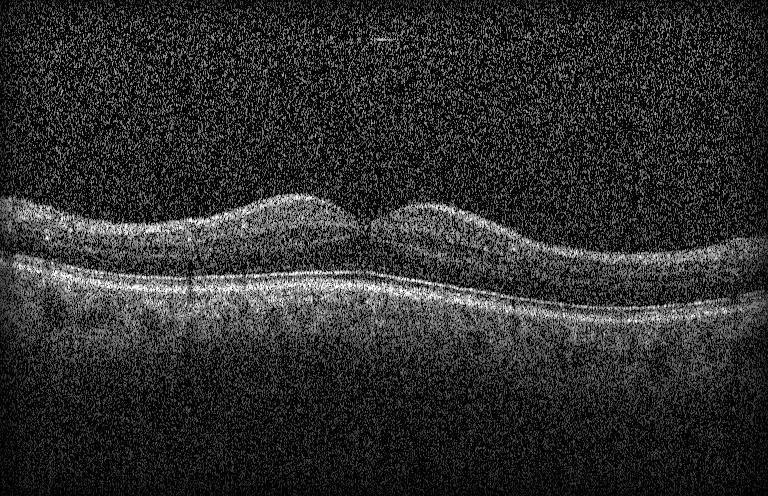
Optical coherence tomography scan. Diagnosis: no CNV, no DME, and no drusen.